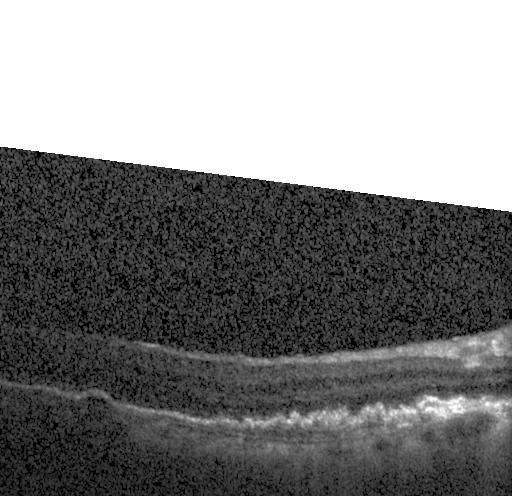

Macular OCT: a choroidal neovascular membrane.